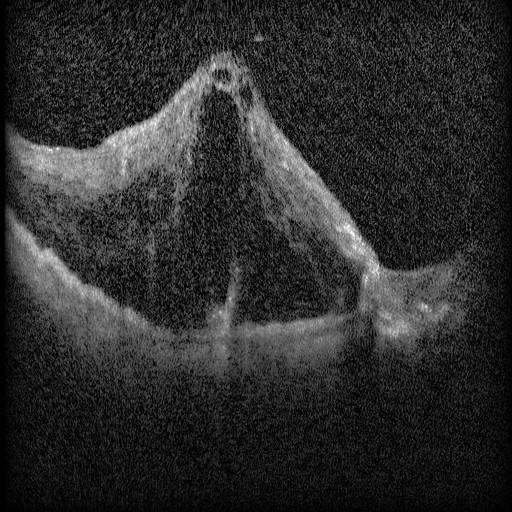
Optical coherence tomography B-scan — Impression: DME.